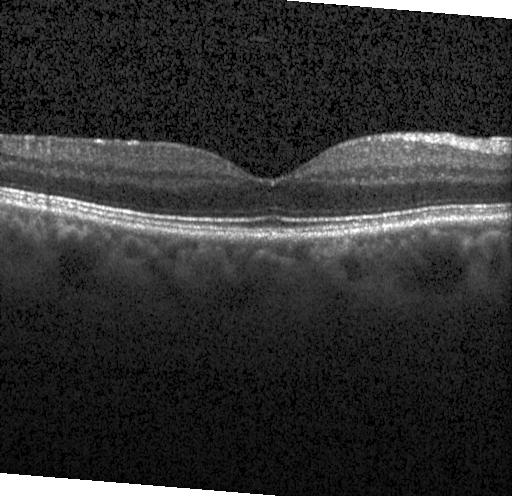 Retinal OCT B-scan
The scan shows neither CNV, DME, nor drusen.